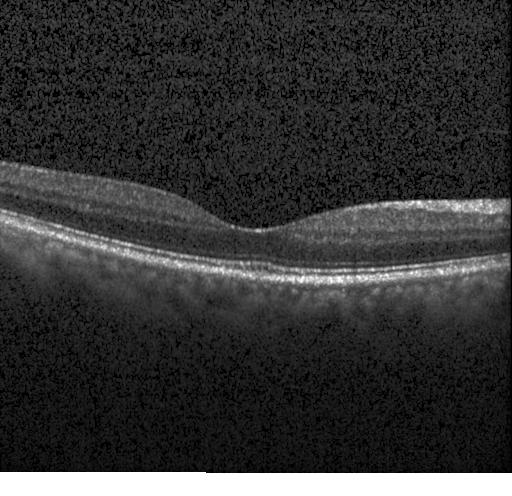
Impression: no CNV, no DME, and no drusen.